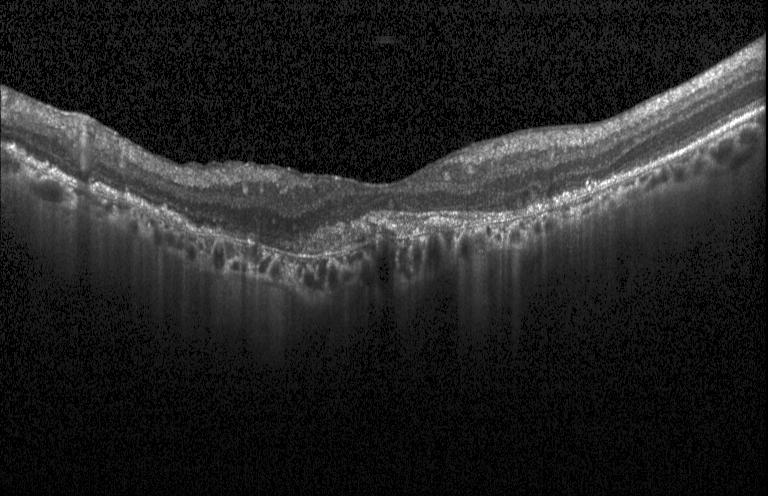

Horizontal scan through the fovea, retinal OCT B-scan, Heidelberg Spectralis, spectral-domain optical coherence tomography — This B-scan demonstrates choroidal neovascularization.